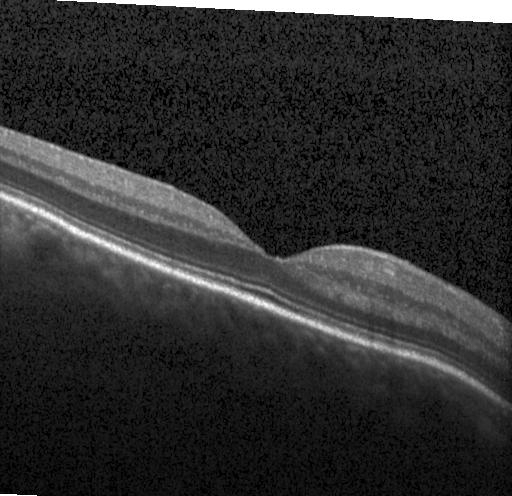
OCT B-scan, SD-OCT. No CNV, DME, or drusen.